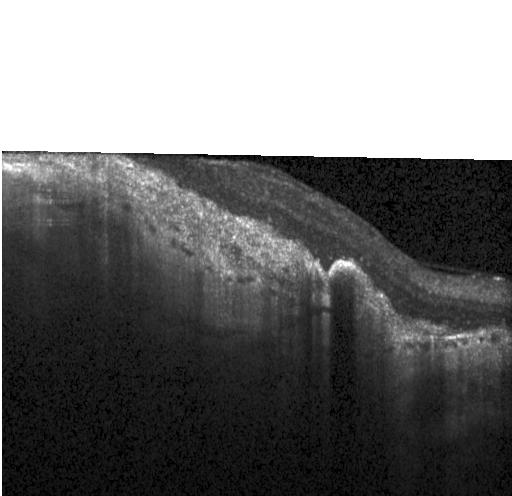
The scan shows a choroidal neovascular membrane.